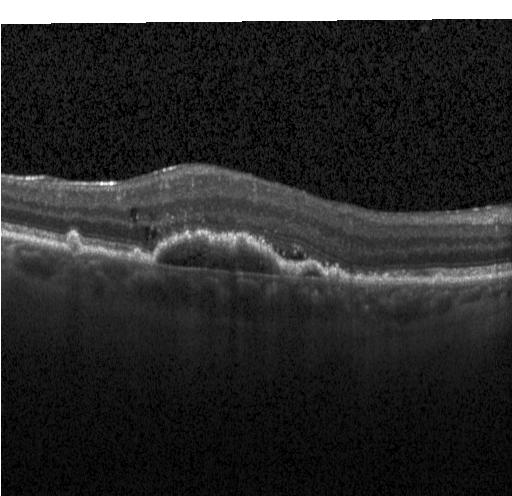
Diagnosis: choroidal neovascularization.